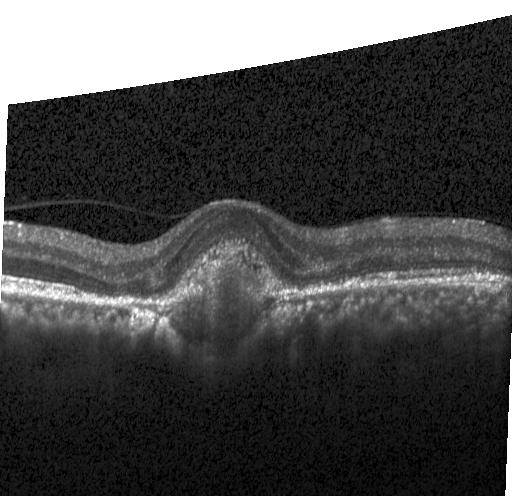 Horizontal scan through the fovea · optical coherence tomography scan · acquired on a Heidelberg Spectralis. OCT finding: choroidal neovascularization (CNV).